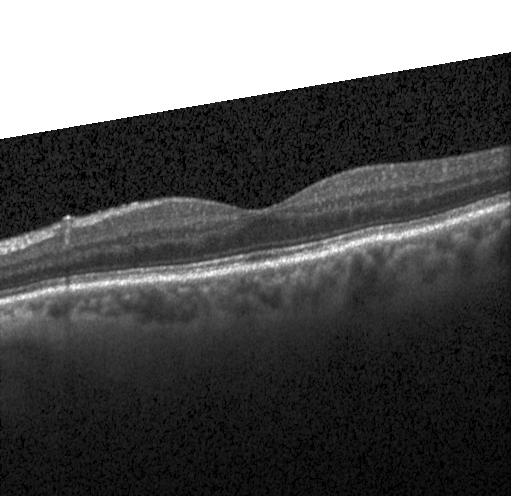 Through the macula · spectral-domain optical coherence tomography · retinal OCT B-scan · Heidelberg Spectralis OCT system. Impression: no evidence of choroidal neovascularization, diabetic macular edema, or drusen.